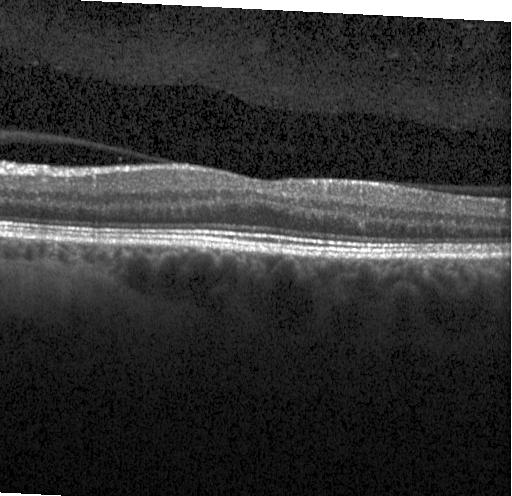
Retinal OCT cross-section showing neither choroidal neovascularization, diabetic macular edema, nor drusen.